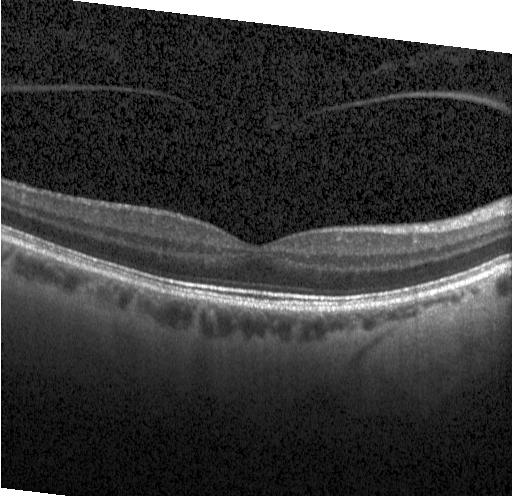

Optical coherence tomography B-scan — Diagnosis: no choroidal neovascularization, no diabetic macular edema, and no drusen.